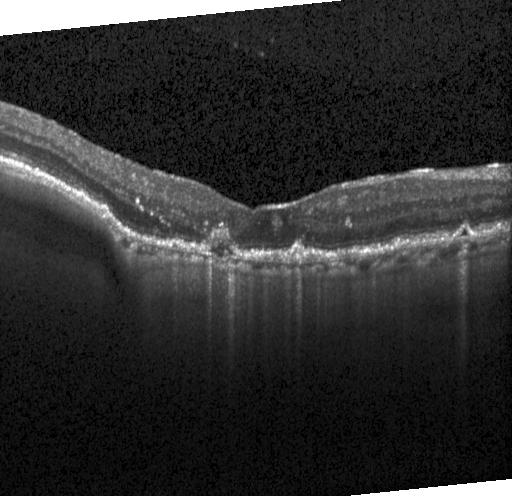 Impression: choroidal neovascularization (CNV).